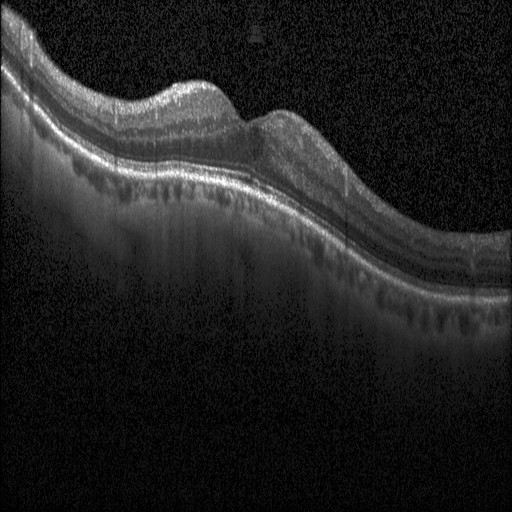

Macular scan, spectral-domain optical coherence tomography, OCT B-scan — Finding: diabetic macular edema (DME).